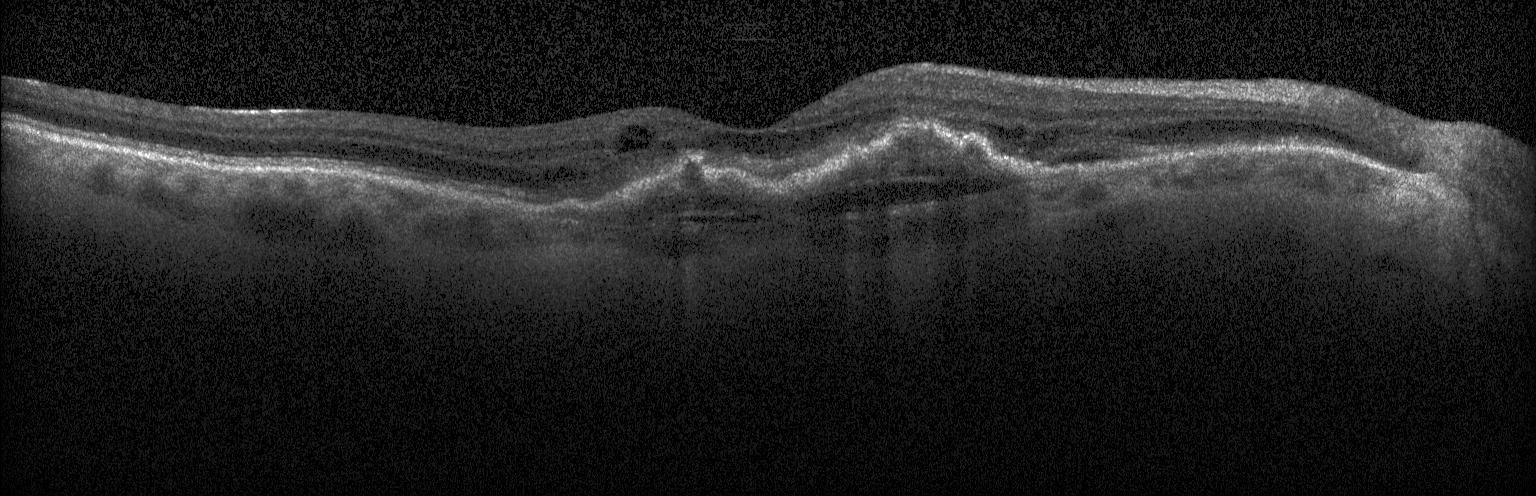 Optical coherence tomography scan
Diagnosis: a choroidal neovascular membrane.